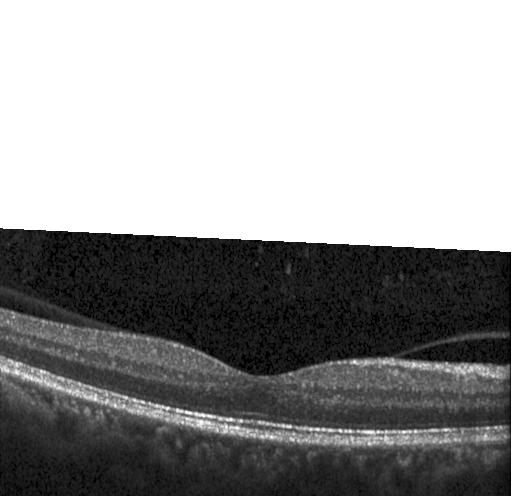 OCT line scan, centered on the fovea
Diagnosis: neither CNV, DME, nor drusen.